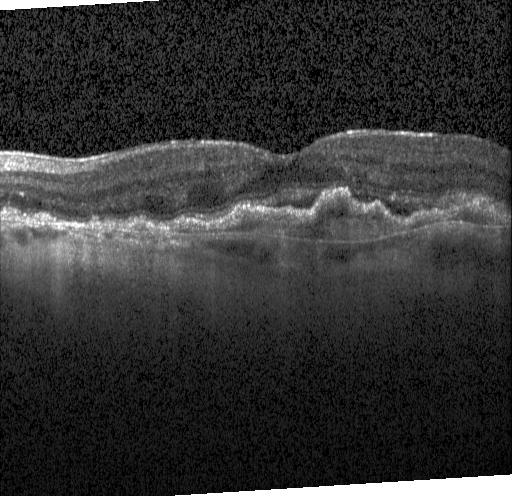

Macular OCT: a choroidal neovascular membrane.